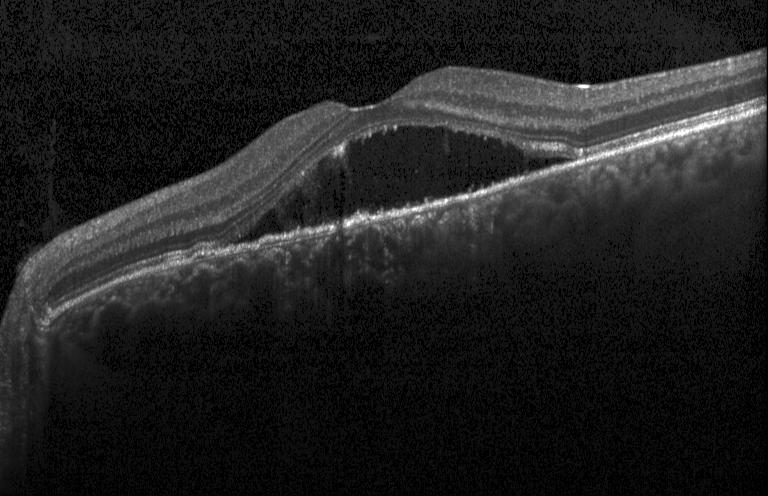

SD-OCT; fovea-centered; optical coherence tomography scan; Heidelberg Spectralis. Impression: a choroidal neovascular membrane.